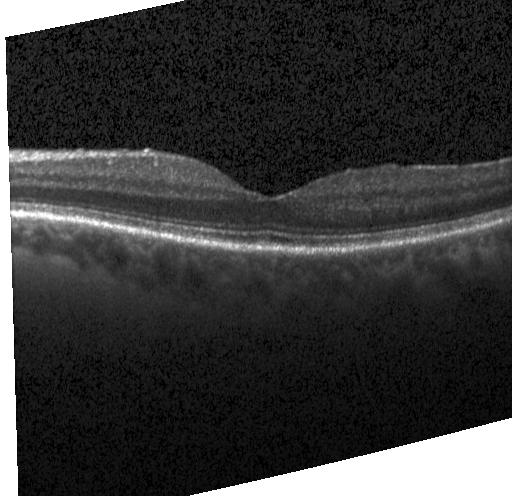

Macular OCT demonstrating no evidence of choroidal neovascularization, diabetic macular edema, or drusen.